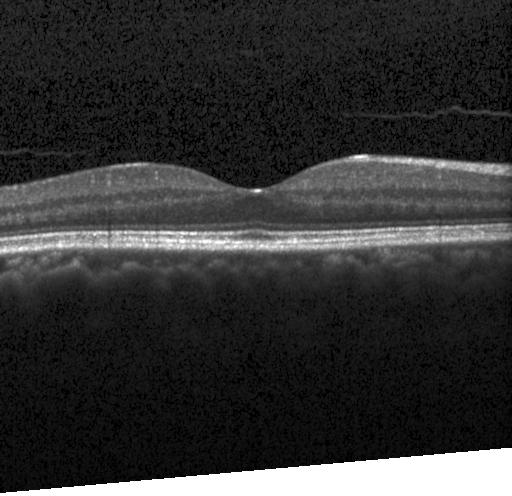

Impression: neither CNV, DME, nor drusen.